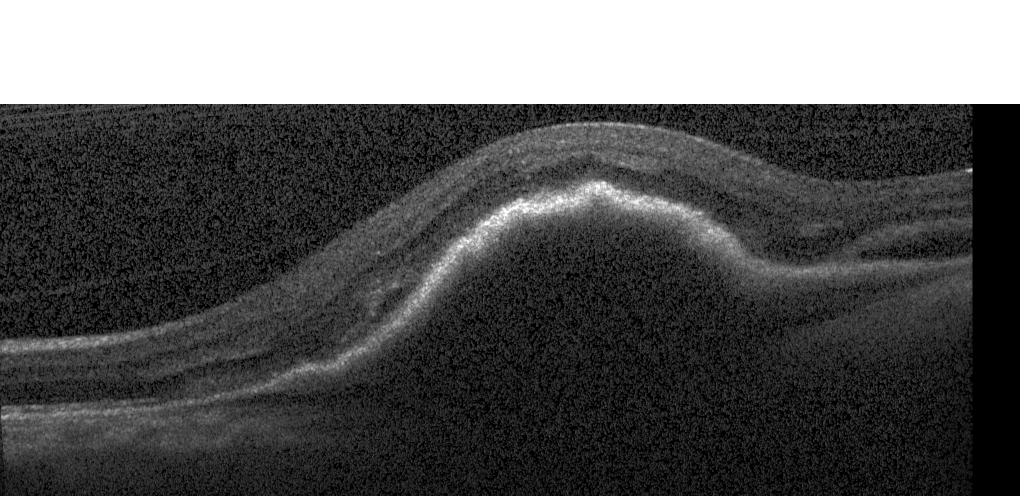

Dx: a choroidal neovascular membrane.